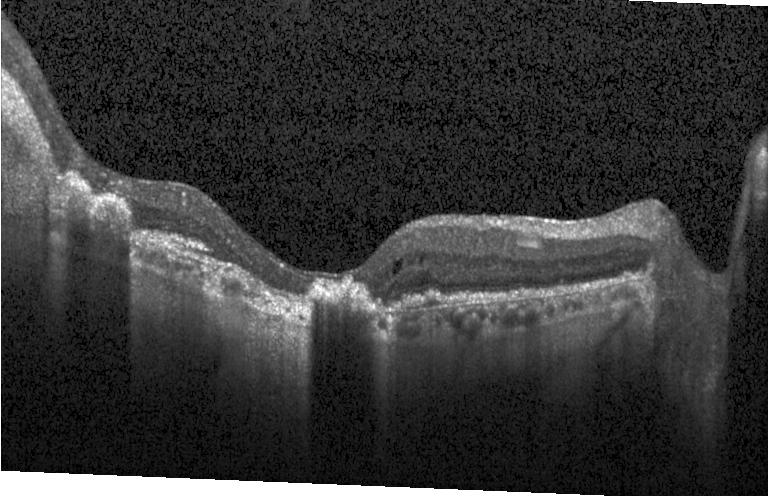

Retinal OCT B-scan.
OCT finding: a choroidal neovascular membrane.